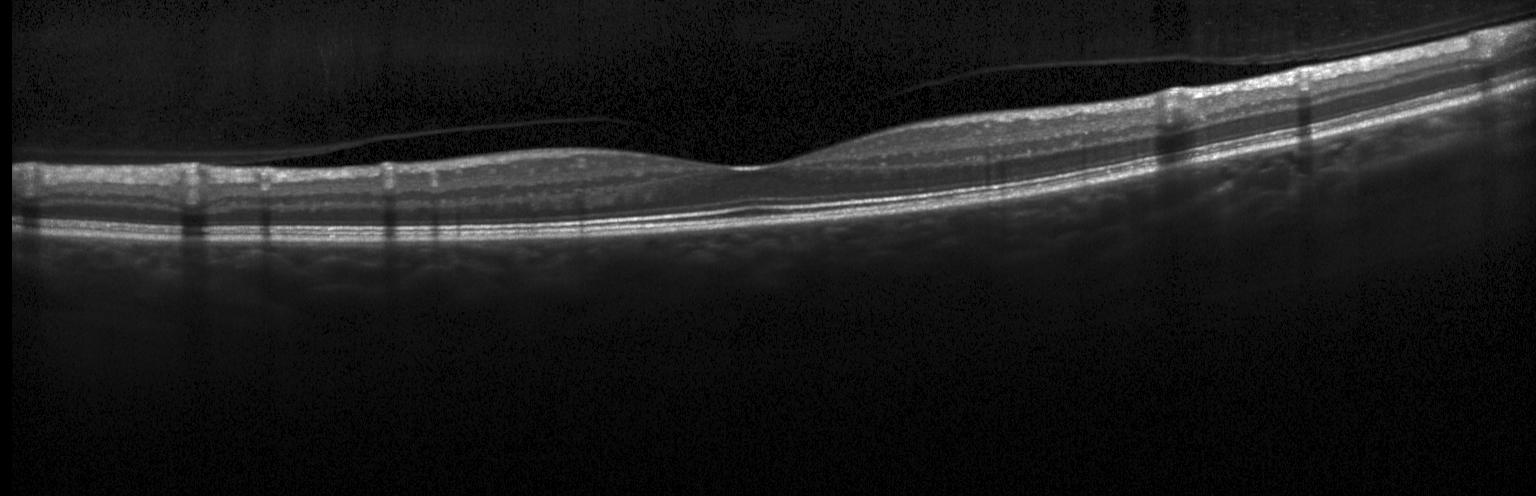

Finding: neither CNV, DME, nor drusen.